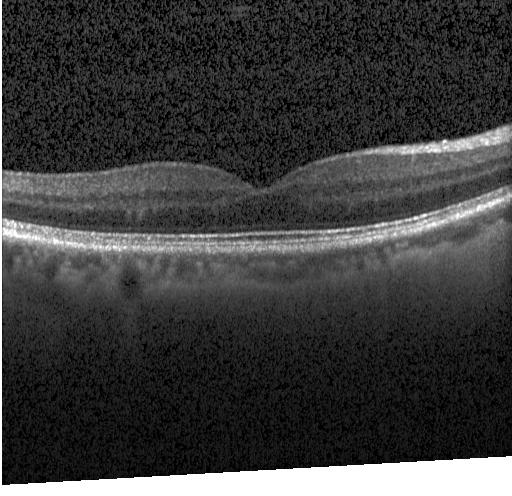 Retinal OCT B-scan. Spectral-domain OCT. Diagnosis: no CNV, no DME, and no drusen.